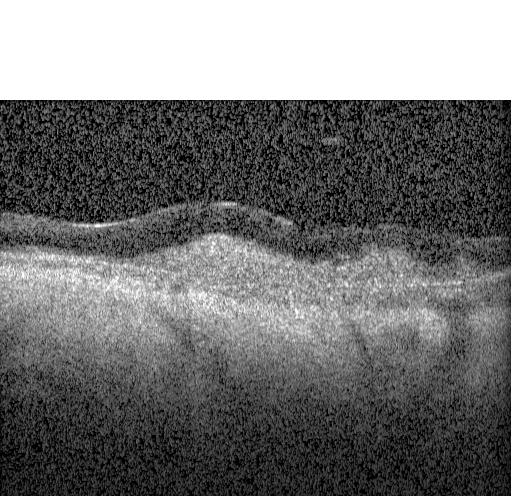
Retinal OCT cross-section showing a choroidal neovascular membrane.